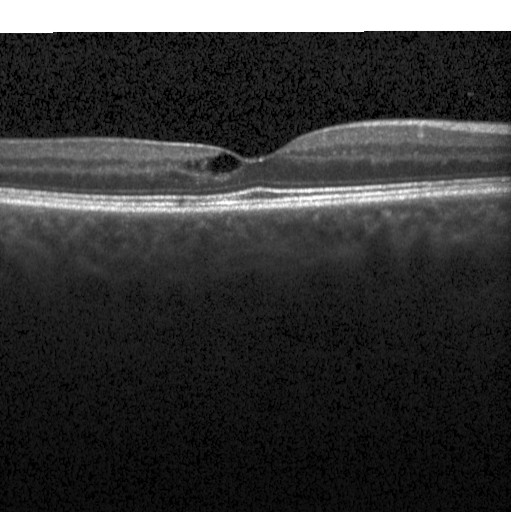 Retinal OCT B-scan; spectral-domain OCT; centered on the fovea; Heidelberg Spectralis — Dx: diabetic macular edema.